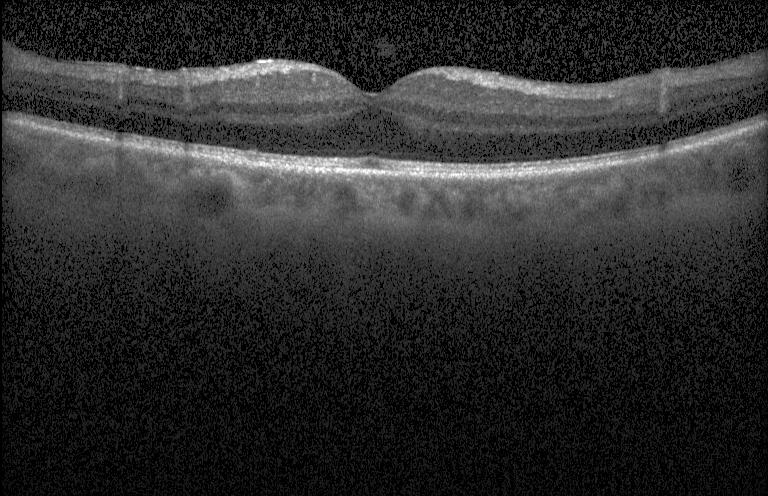
No evidence of choroidal neovascularization, diabetic macular edema, or drusen.